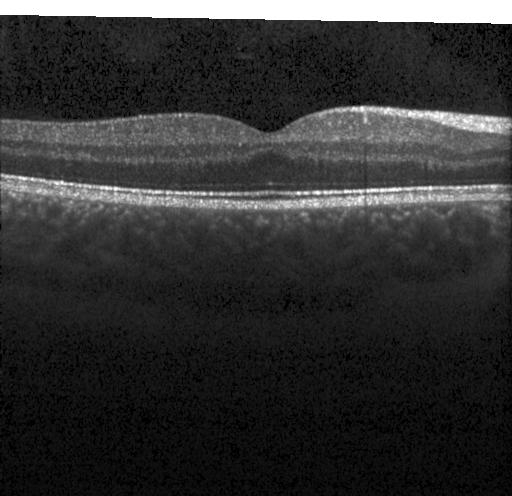

Through the macula · optical coherence tomography scan
This B-scan demonstrates neither choroidal neovascularization, diabetic macular edema, nor drusen.